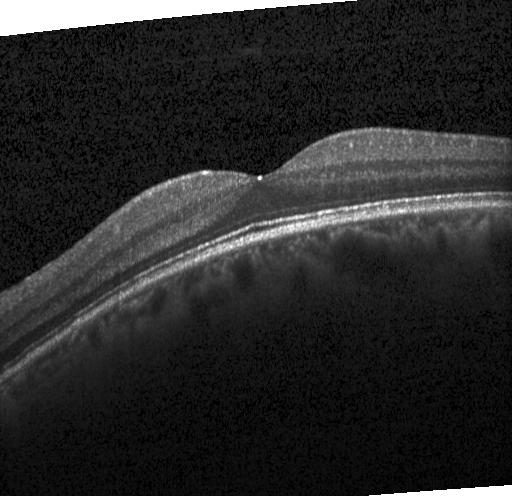
OCT B-scan. Heidelberg Spectralis OCT system — This B-scan demonstrates no evidence of CNV, DME, or drusen.